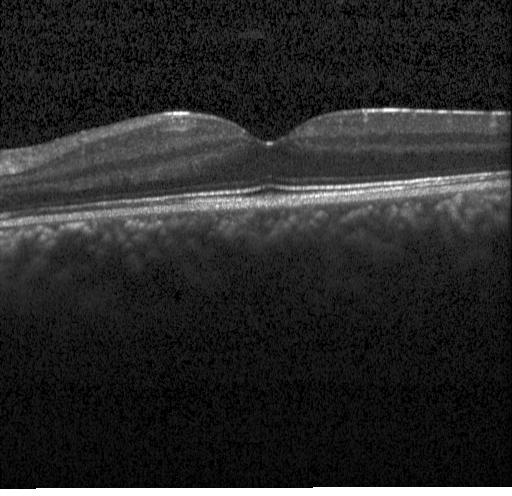
Retinal OCT B-scan. Finding: no choroidal neovascularization, no diabetic macular edema, and no drusen.